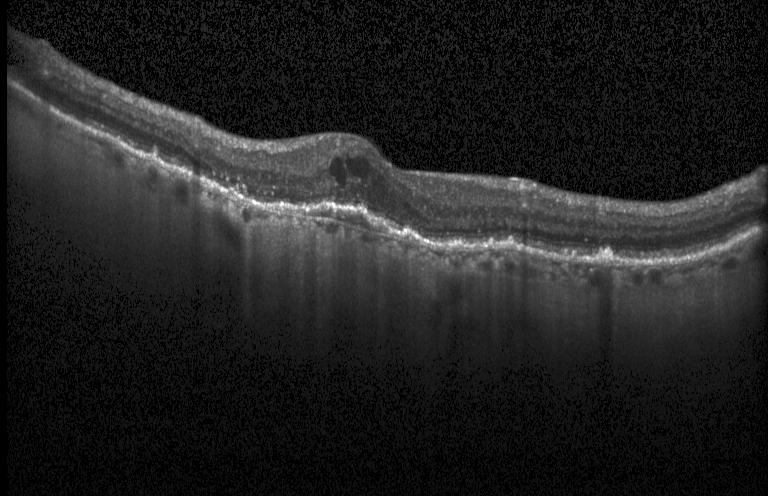
This B-scan demonstrates a choroidal neovascular membrane.